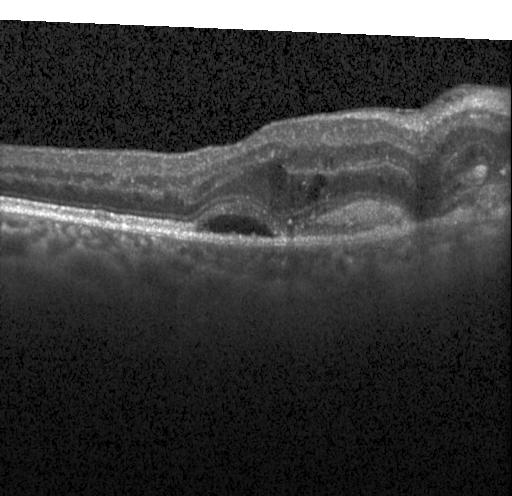 OCT scan showing choroidal neovascularization (CNV).